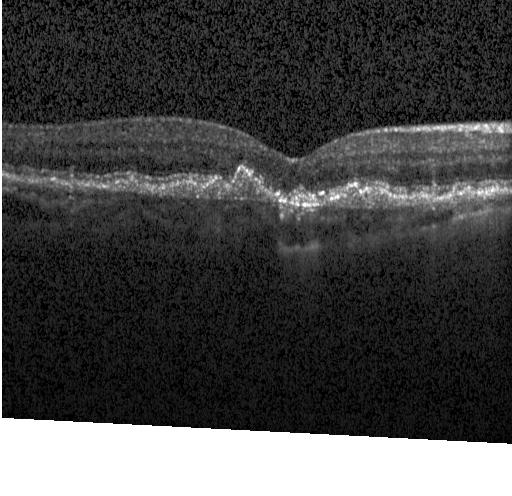

SD-OCT; OCT line scan; instrument: Heidelberg Spectralis; through the macula
Diagnosis: choroidal neovascularization.